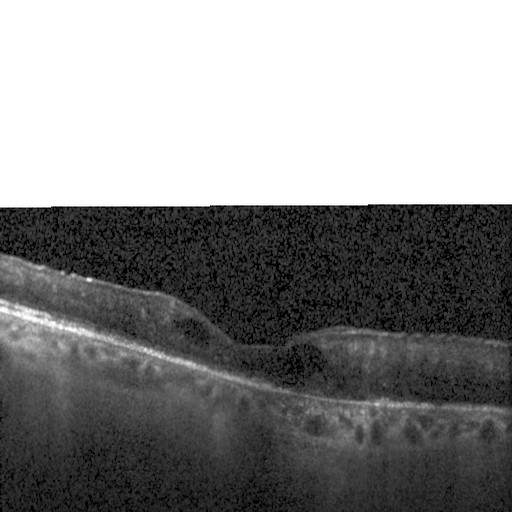 Spectral-domain OCT · optical coherence tomography B-scan · instrument: Heidelberg Spectralis
Finding: DME.